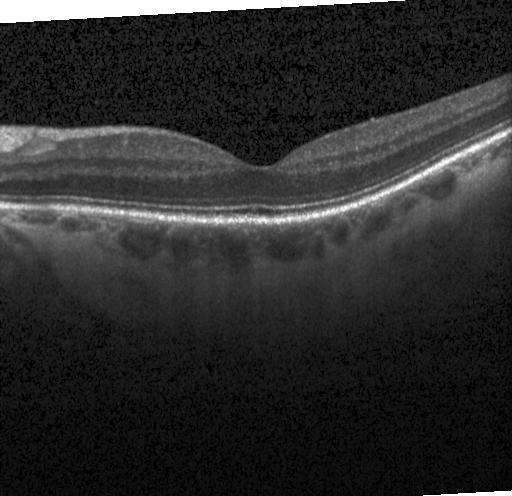 Finding: no choroidal neovascularization, no diabetic macular edema, and no drusen.